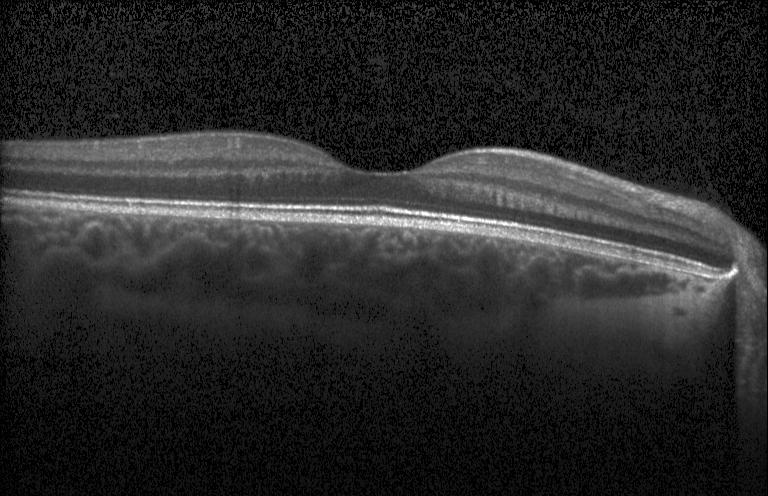
Optical coherence tomography B-scan.
Finding: no evidence of CNV, DME, or drusen.